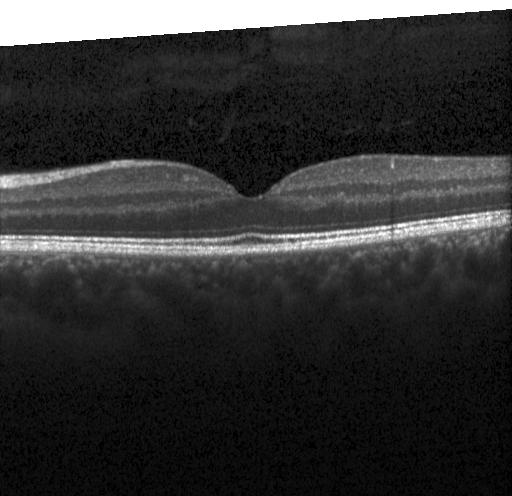
Centered on the fovea, spectral-domain OCT, optical coherence tomography B-scan, Heidelberg Spectralis — Impression: neither choroidal neovascularization, diabetic macular edema, nor drusen.